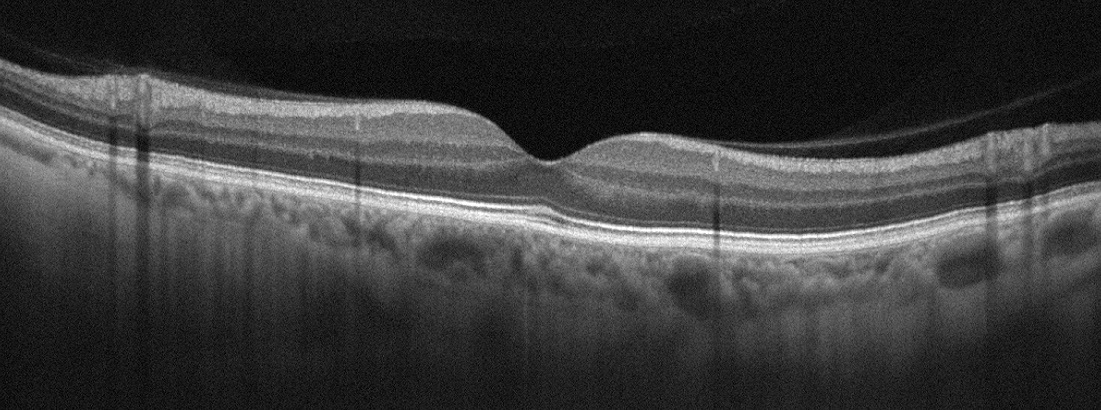

Optovue Avanti RTVue XR, retinal OCT cross-section, fovea-centered.
Diagnosis: absence of AMD, DME, ERM, RAO, RVO, and vitreomacular interface disease.